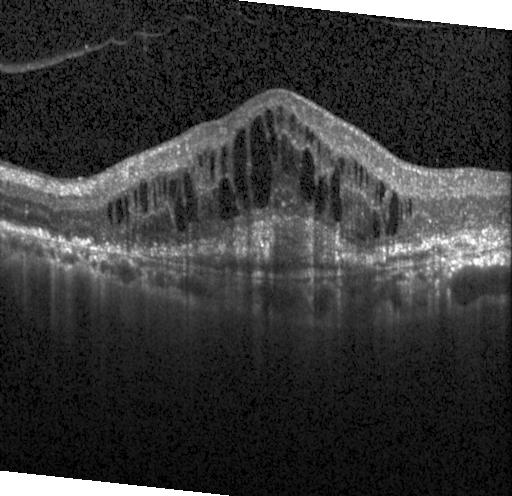 Acquired on a Heidelberg Spectralis; OCT B-scan; spectral-domain OCT. Diagnosis: choroidal neovascularization.